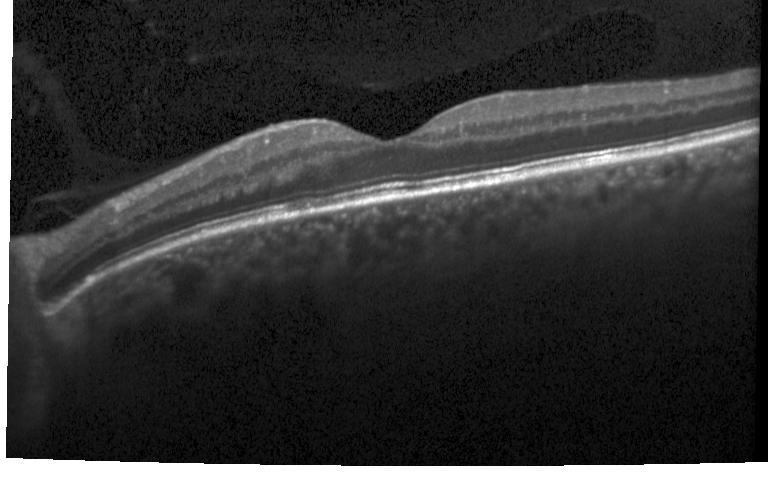

Impression: no choroidal neovascularization, no diabetic macular edema, and no drusen.